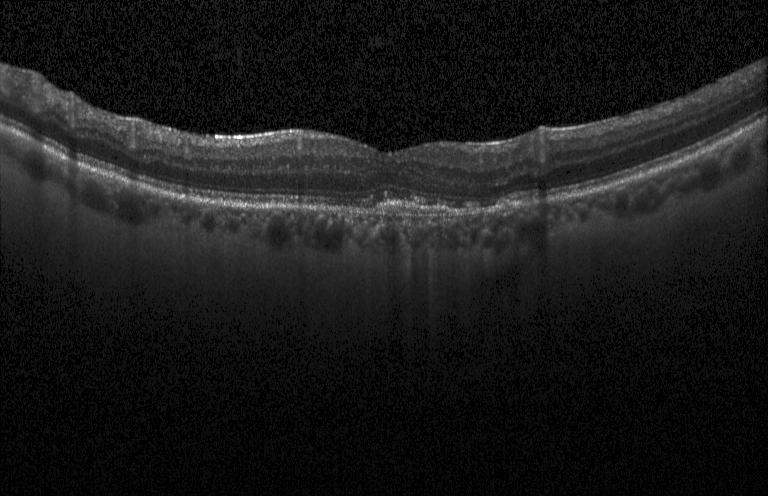 Diagnosis: choroidal neovascularization (CNV).